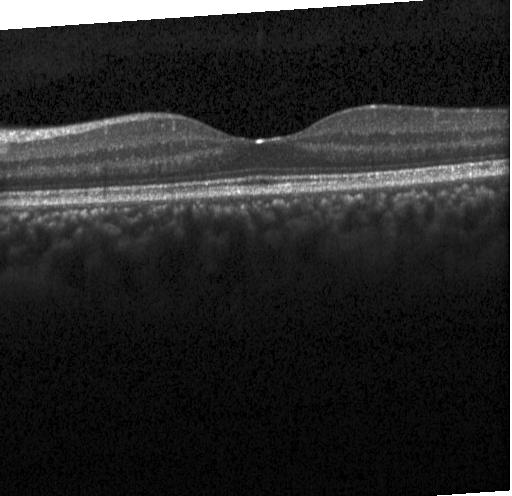
Impression: no evidence of choroidal neovascularization, diabetic macular edema, or drusen.